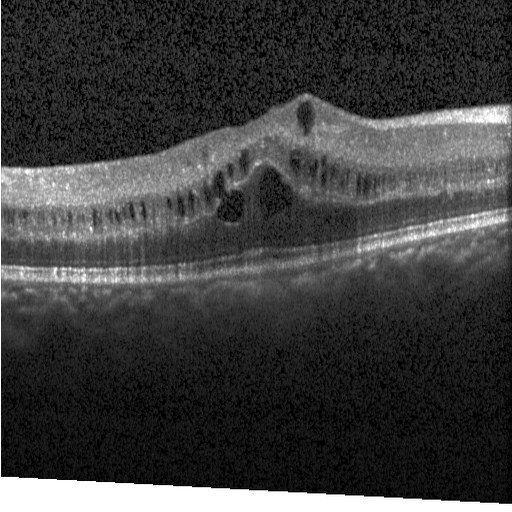

Macular OCT demonstrating diabetic macular edema.